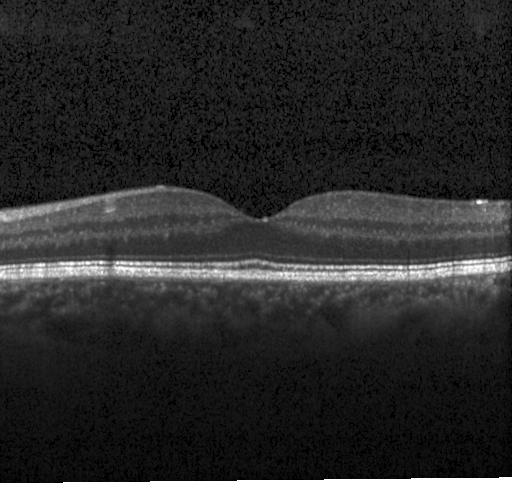

Instrument: Heidelberg Spectralis, OCT B-scan. Diagnosis: no CNV, DME, or drusen.